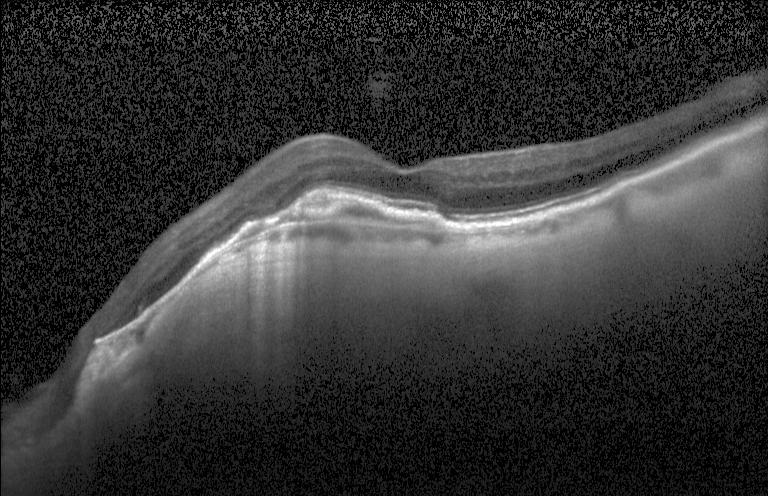

Retinal OCT cross-section. Diagnosis: CNV.